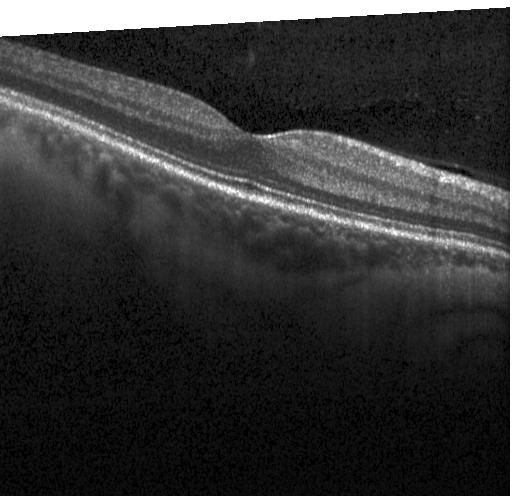
Spectral-domain OCT. Horizontal scan through the fovea. Retinal OCT cross-section.
Dx: no choroidal neovascularization, no diabetic macular edema, and no drusen.